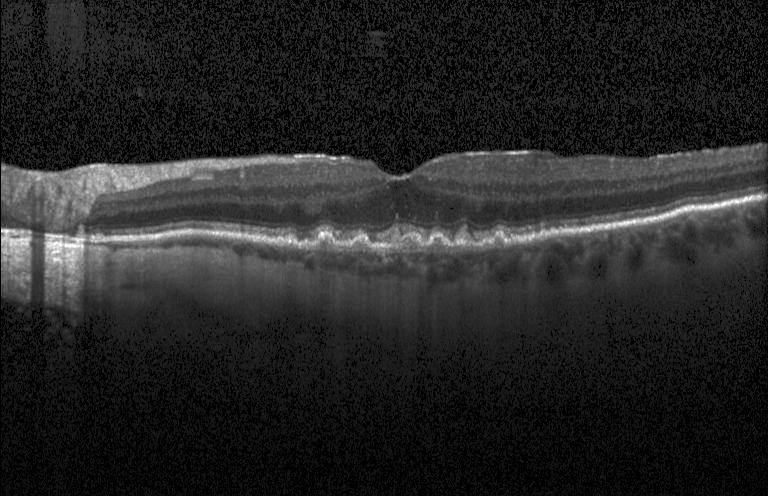
Impression: sub-RPE drusenoid deposits.